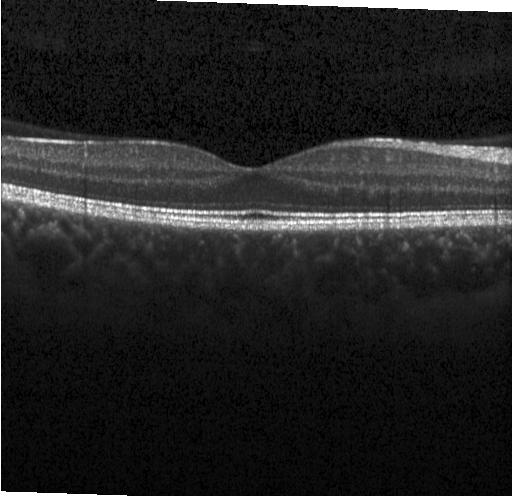
Impression: no evidence of CNV, DME, or drusen.